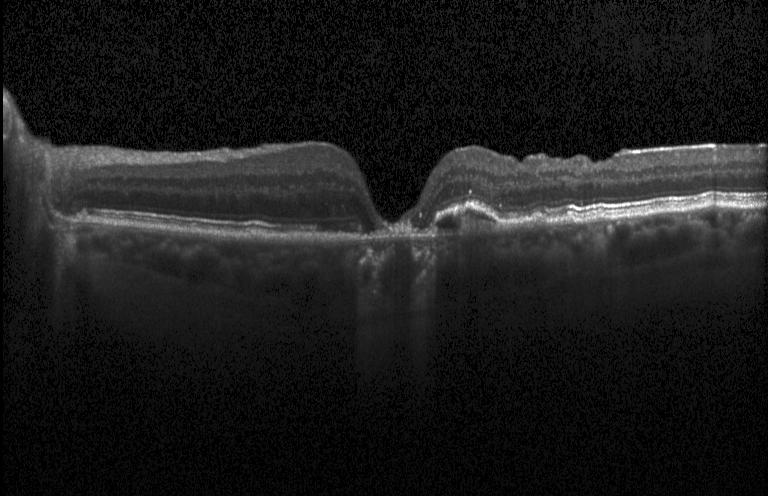

OCT B-scan showing CNV.